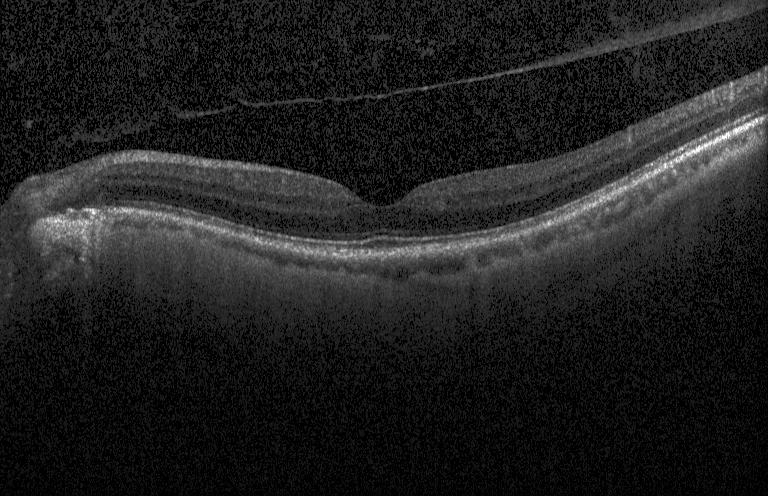

Impression: no CNV, DME, or drusen.